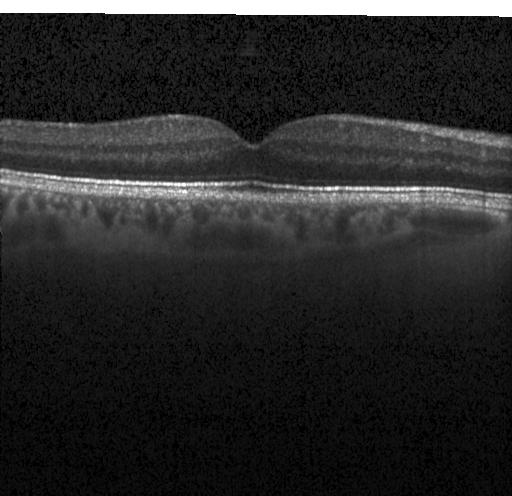

OCT B-scan.
Diagnosis: no CNV, DME, or drusen.